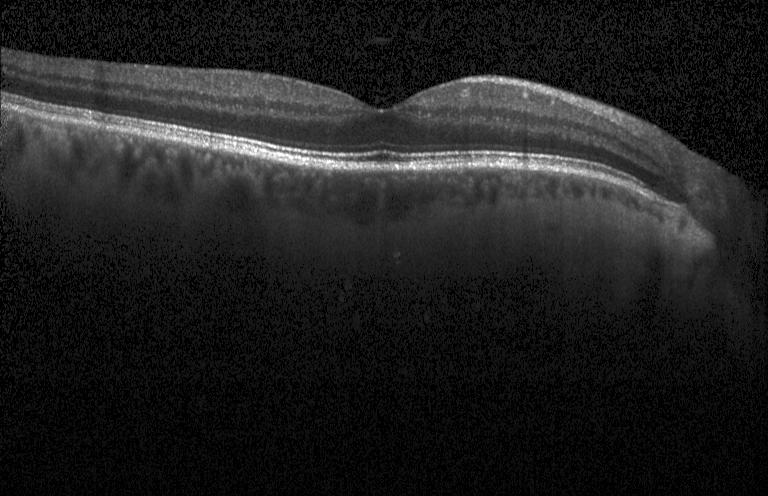 Acquired on a Heidelberg Spectralis, horizontal scan through the fovea, retinal OCT cross-section, spectral-domain OCT — No choroidal neovascularization, no diabetic macular edema, and no drusen.